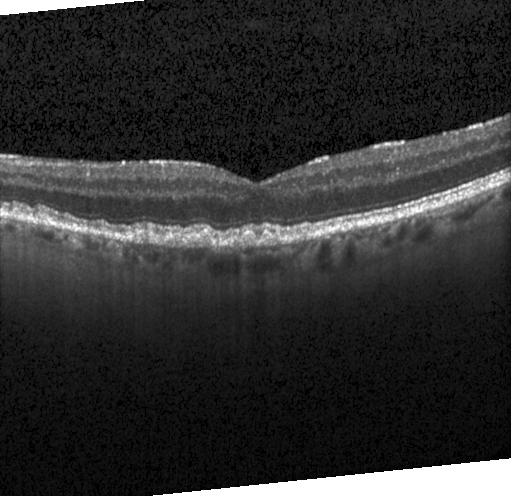

OCT scan showing sub-RPE drusenoid deposits.